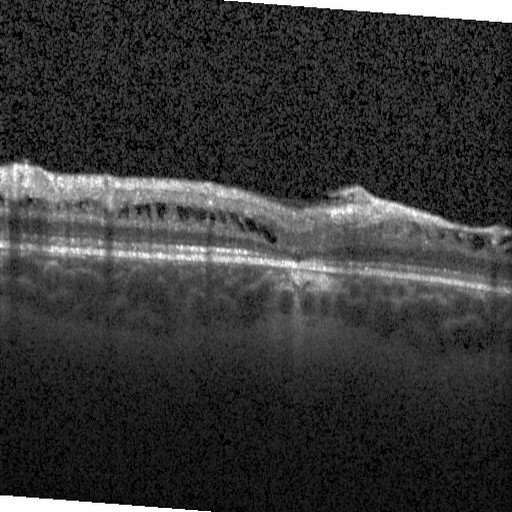
OCT B-scan.
OCT finding: diabetic macular edema.